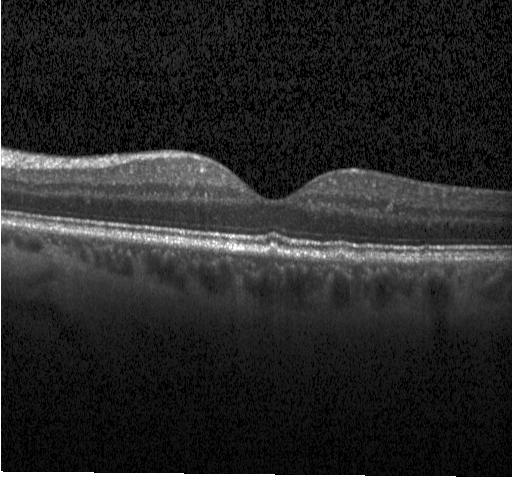 Fovea-centered · Heidelberg Spectralis OCT system · retinal OCT cross-section · spectral-domain OCT
This B-scan demonstrates drusen.